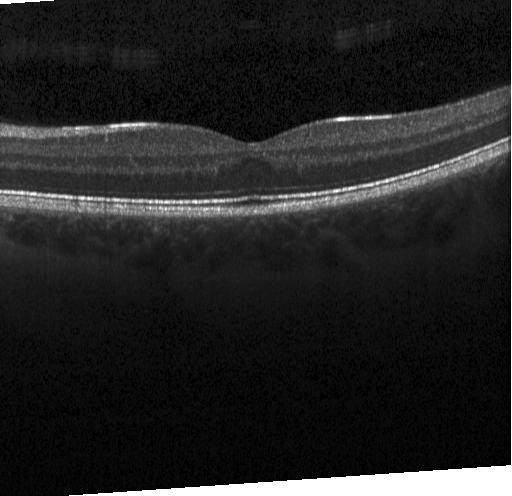

OCT B-scan, spectral-domain optical coherence tomography, Heidelberg Spectralis, fovea-centered.
OCT finding: no choroidal neovascularization, diabetic macular edema, or drusen.